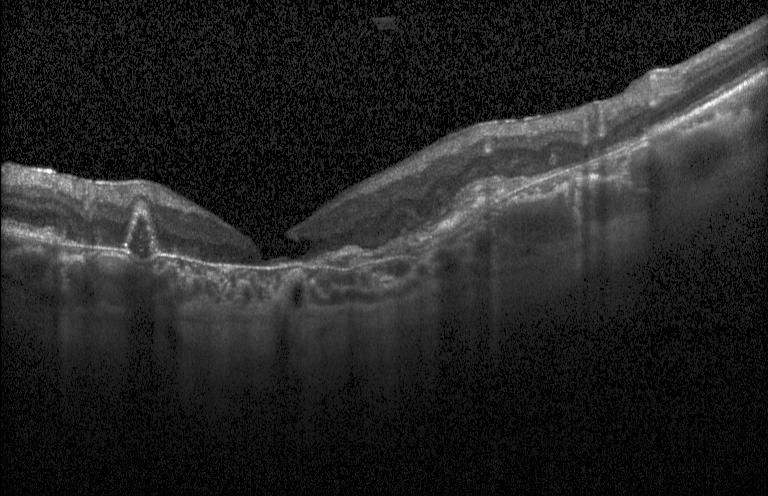 Retinal OCT cross-section.
Dx: choroidal neovascularization (CNV).